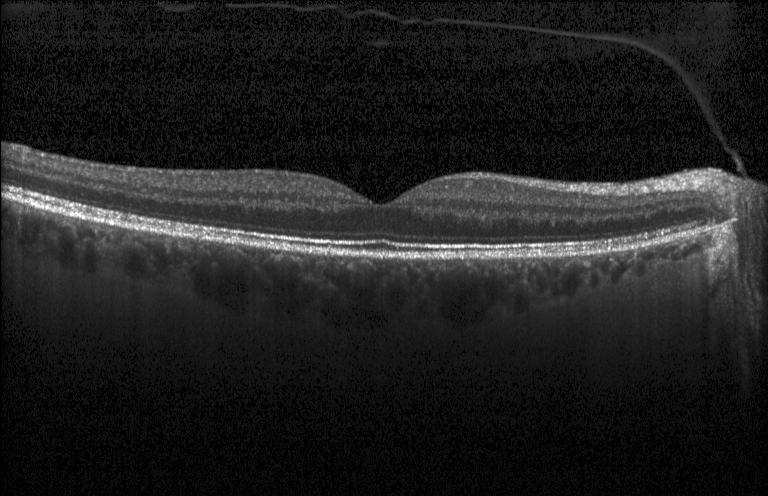 Through the macula, OCT B-scan
Diagnosis: no choroidal neovascularization, diabetic macular edema, or drusen.